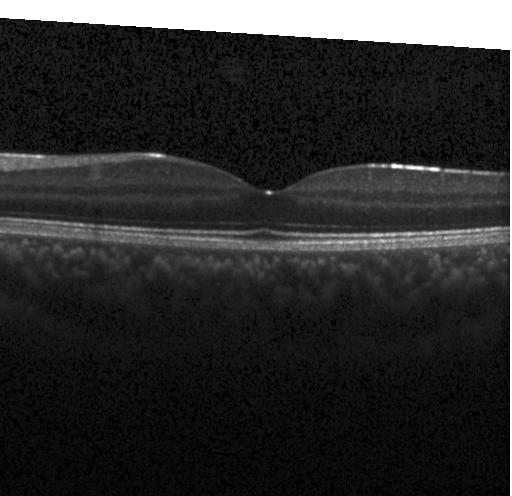
Acquired on a Heidelberg Spectralis, optical coherence tomography B-scan
Diagnosis: no choroidal neovascularization, no diabetic macular edema, and no drusen.